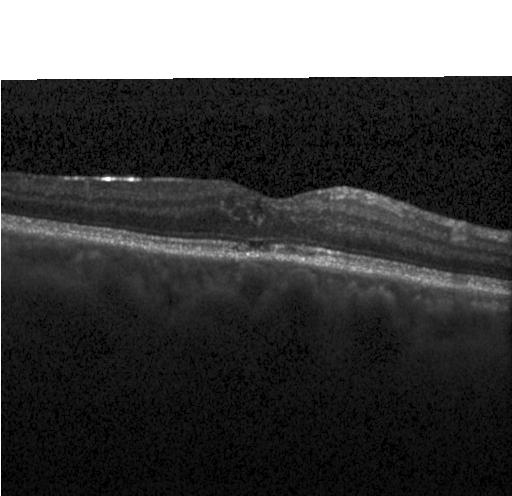

Retinal OCT B-scan · fovea-centered · instrument: Heidelberg Spectralis
Finding: diabetic macular edema.